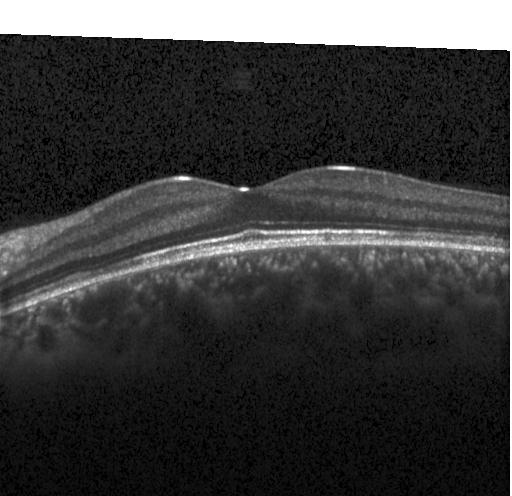

Diagnosis: no evidence of CNV, DME, or drusen.